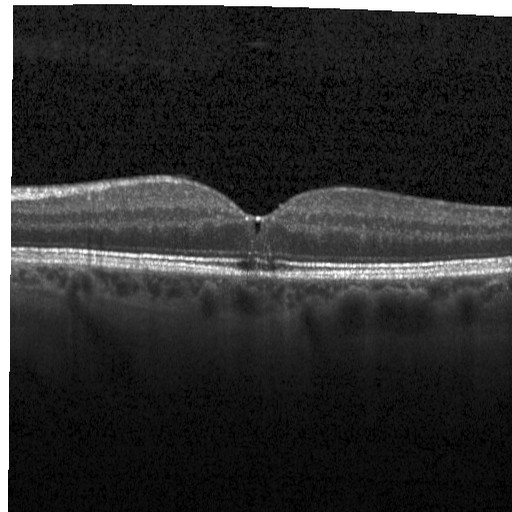 Through the macula, OCT B-scan.
Finding: diabetic macular edema.